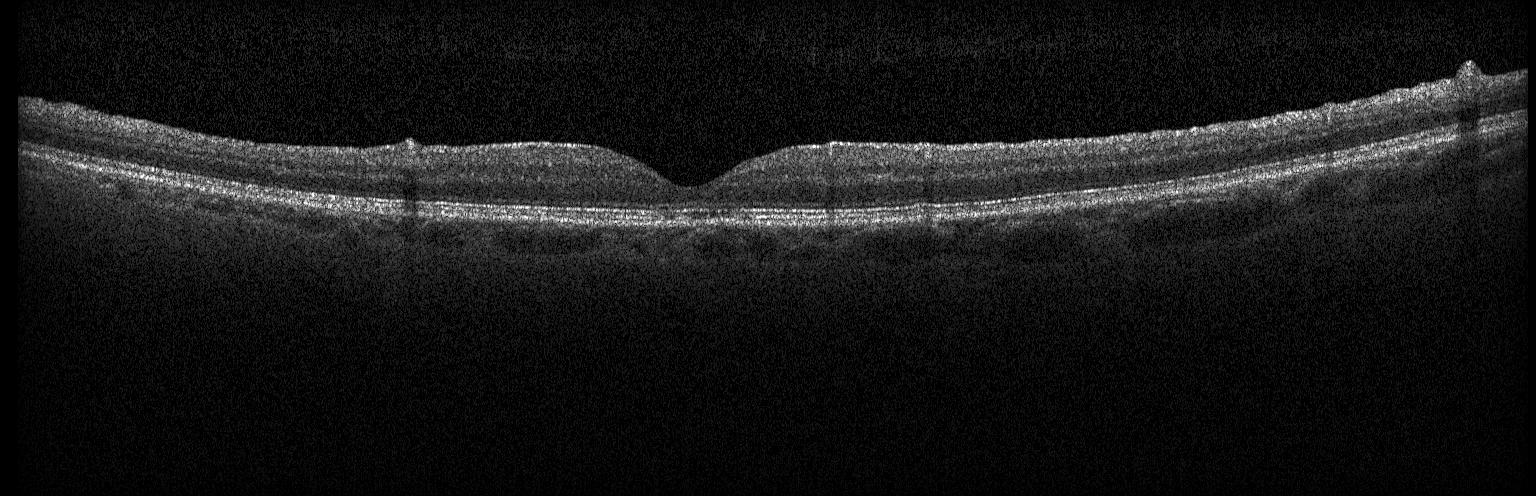 Diagnosis: no choroidal neovascularization, diabetic macular edema, or drusen.